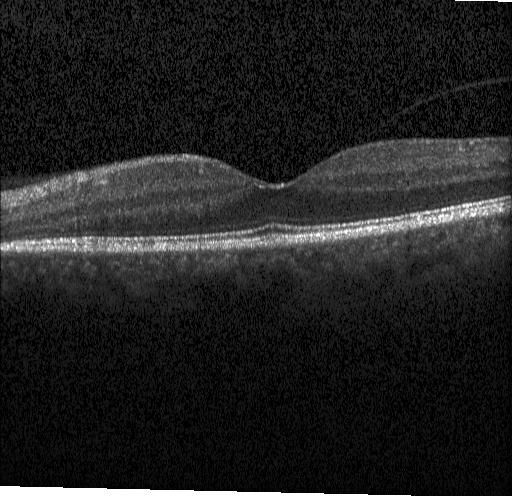
Diagnosis: no choroidal neovascularization, no diabetic macular edema, and no drusen.